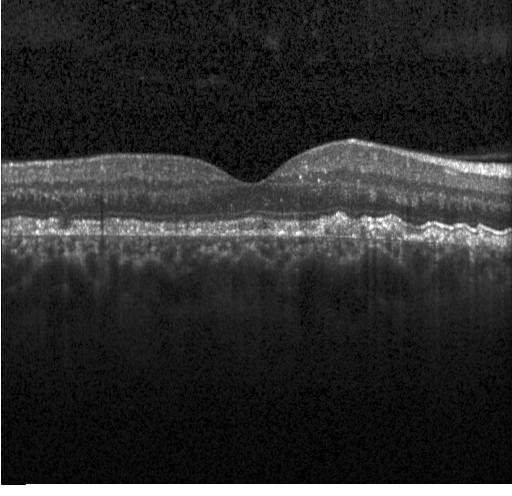
OCT line scan. Instrument: Heidelberg Spectralis. Centered on the fovea. Spectral-domain optical coherence tomography
Finding: sub-RPE drusenoid deposits.